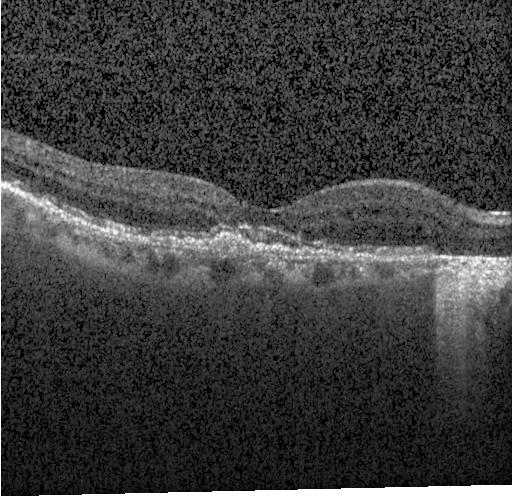

Optical coherence tomography B-scan — The scan shows choroidal neovascularization.